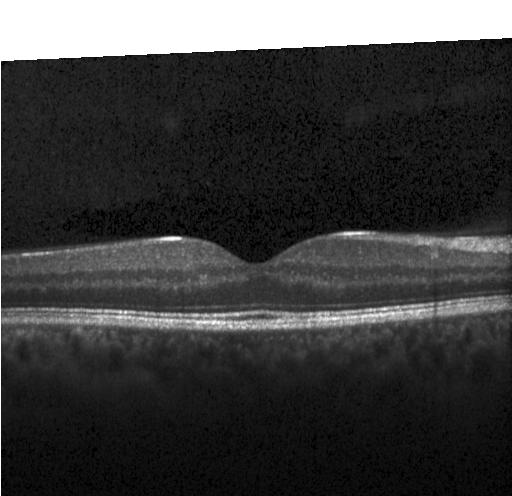 Heidelberg Spectralis · spectral-domain OCT · OCT B-scan
OCT finding: no choroidal neovascularization, no diabetic macular edema, and no drusen.